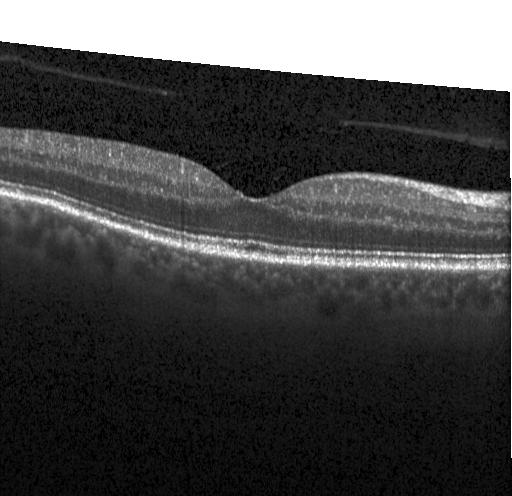
Diagnosis: no evidence of choroidal neovascularization, diabetic macular edema, or drusen.